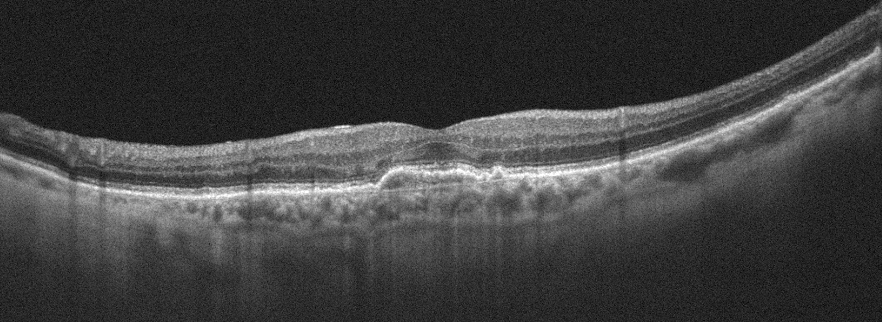

OCT B-scan showing age-related macular degeneration.